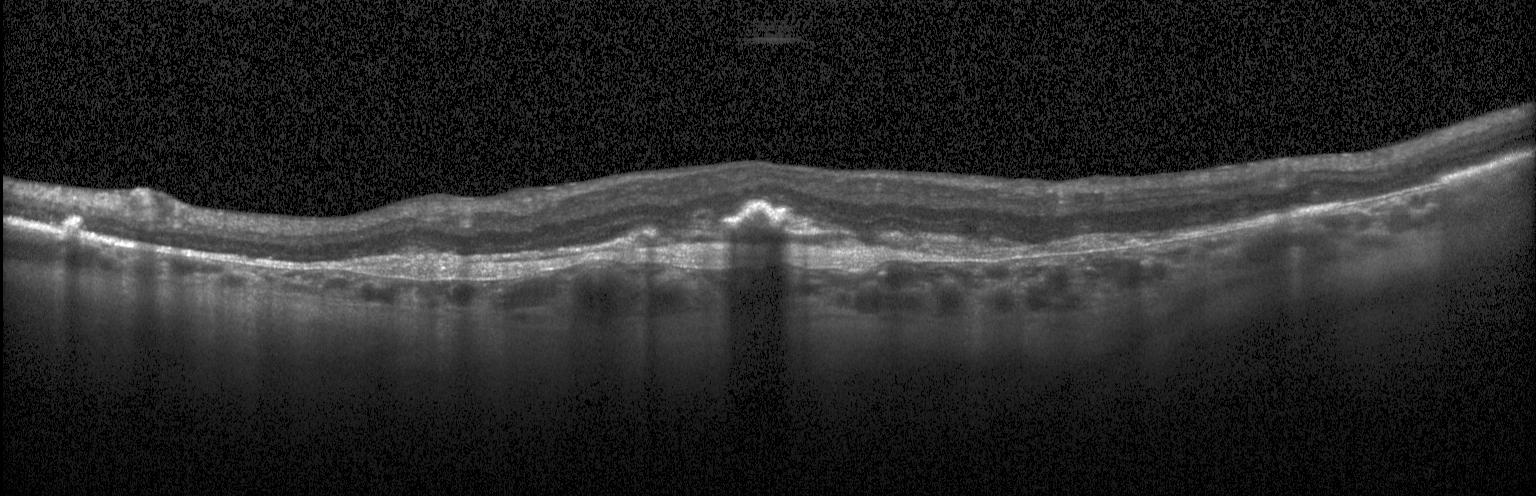 Heidelberg Spectralis OCT system; retinal OCT B-scan; through the macula; spectral-domain optical coherence tomography. Finding: CNV.